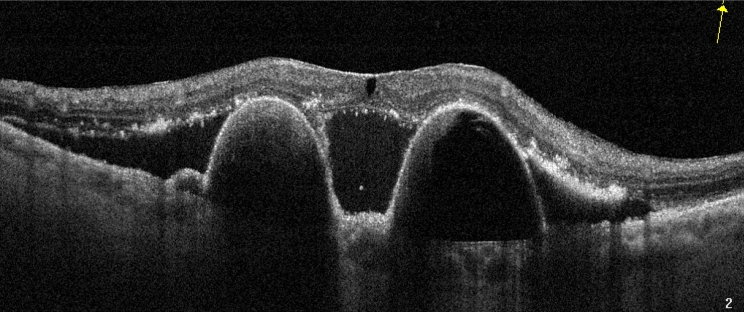
OCT line scan; macular scan
This B-scan demonstrates age-related macular degeneration (AMD).